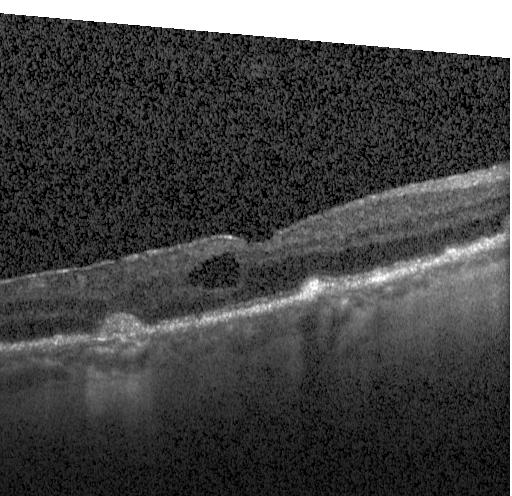
Diagnosis: a choroidal neovascular membrane.